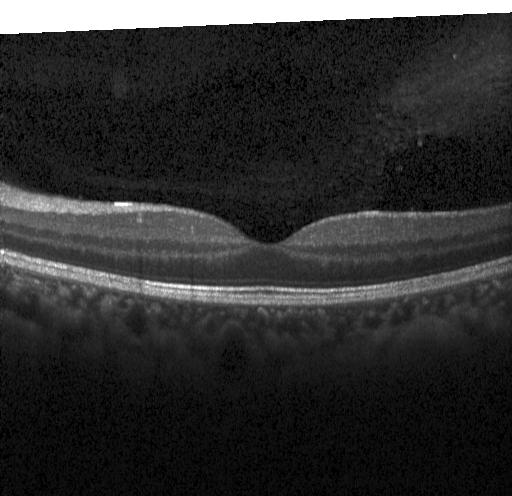

Through the macula · OCT B-scan · spectral-domain optical coherence tomography
OCT finding: no choroidal neovascularization, diabetic macular edema, or drusen.